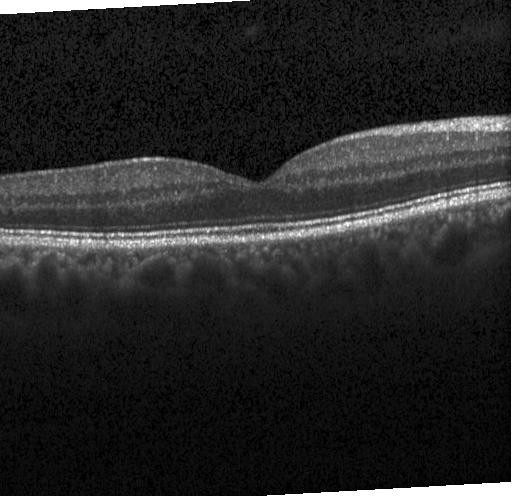
OCT line scan. Instrument: Heidelberg Spectralis. Fovea-centered. Impression: no evidence of choroidal neovascularization, diabetic macular edema, or drusen.